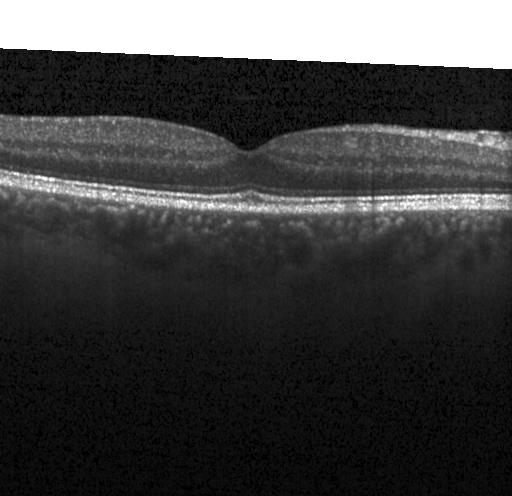
SD-OCT · Heidelberg Spectralis · retinal OCT B-scan. Diagnosis: neither choroidal neovascularization, diabetic macular edema, nor drusen.